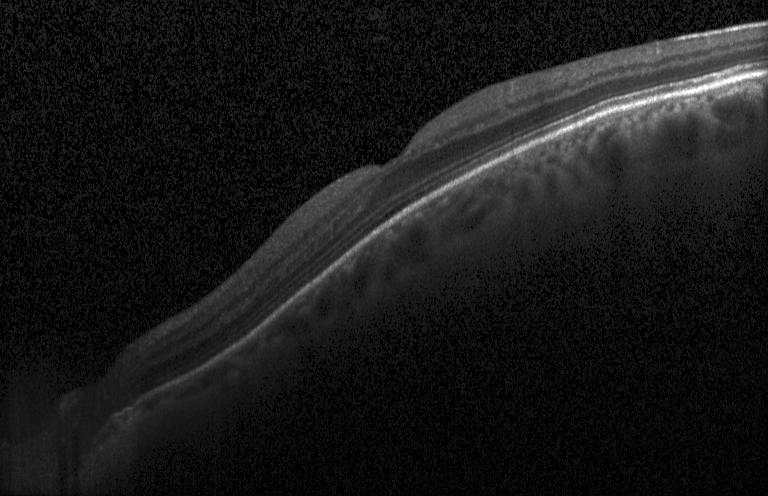

Heidelberg Spectralis · optical coherence tomography B-scan
Impression: neither CNV, DME, nor drusen.